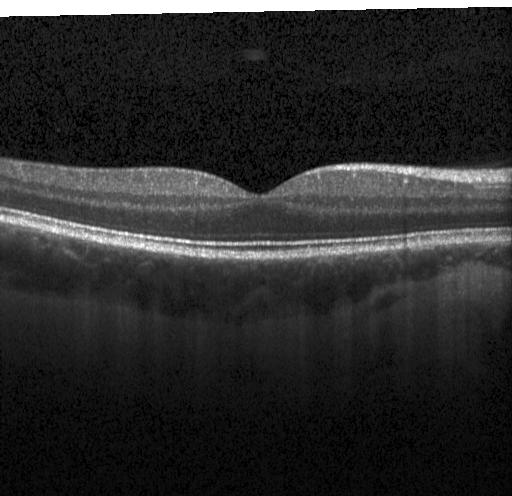
OCT line scan.
The scan shows no evidence of CNV, DME, or drusen.